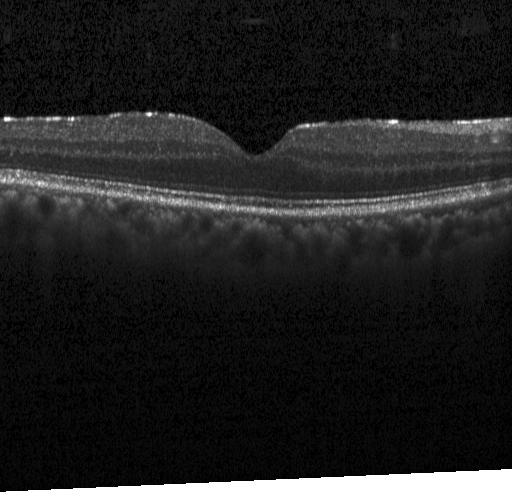
Retinal OCT B-scan. Acquired on a Heidelberg Spectralis. SD-OCT.
Dx: neither CNV, DME, nor drusen.